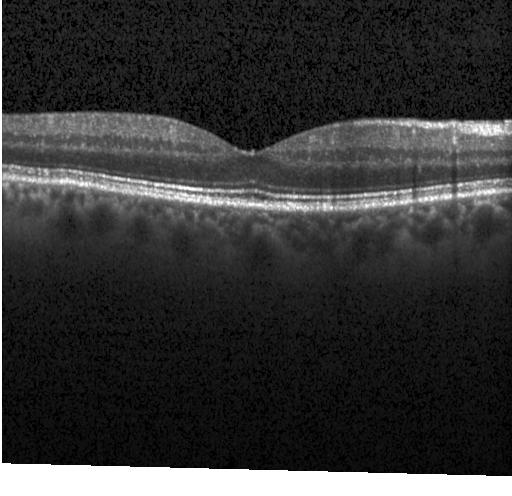 Optical coherence tomography scan; spectral-domain OCT
This B-scan demonstrates no choroidal neovascularization, diabetic macular edema, or drusen.